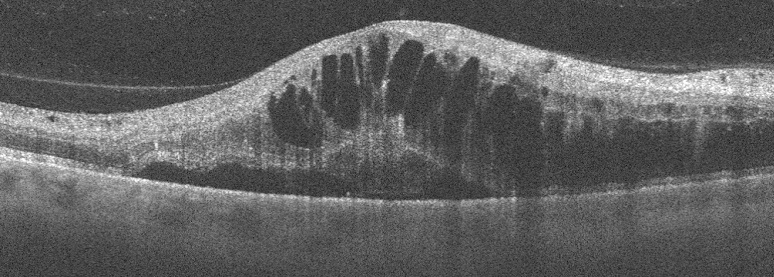

Optovue Avanti RTVue XR. Retinal OCT B-scan — Dx: RVO.